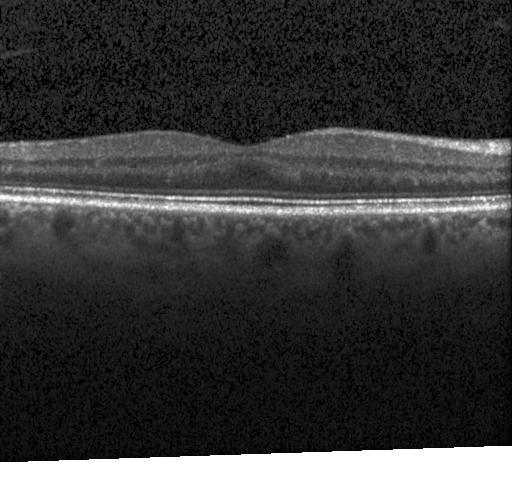

OCT line scan. Instrument: Heidelberg Spectralis.
Assessment: no choroidal neovascularization, diabetic macular edema, or drusen.